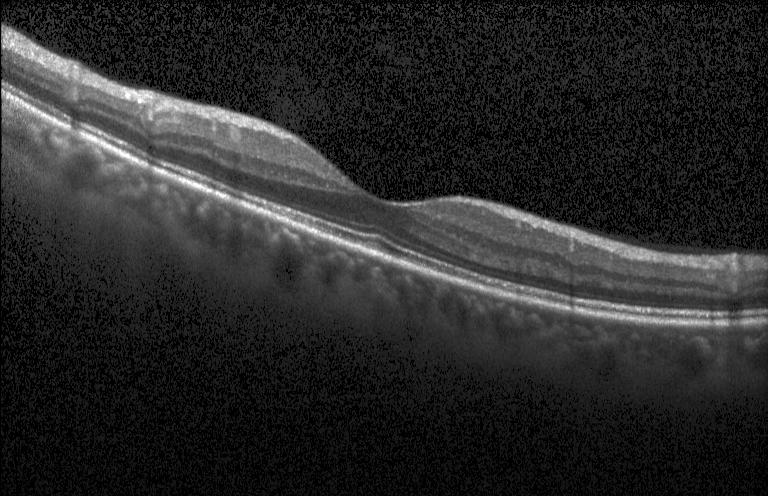
Heidelberg Spectralis · optical coherence tomography scan. Dx: no evidence of CNV, DME, or drusen.